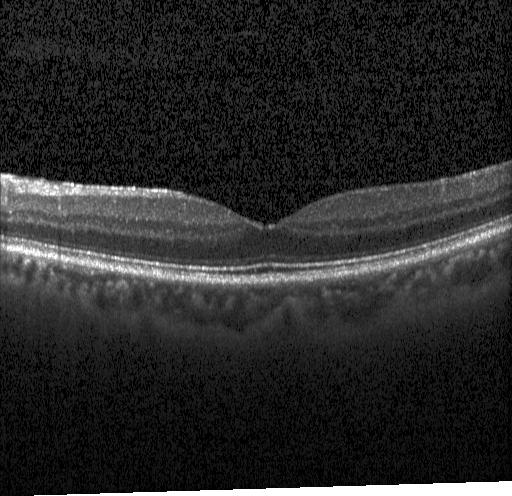

Acquired on a Heidelberg Spectralis, optical coherence tomography scan, spectral-domain optical coherence tomography. OCT finding: neither CNV, DME, nor drusen.